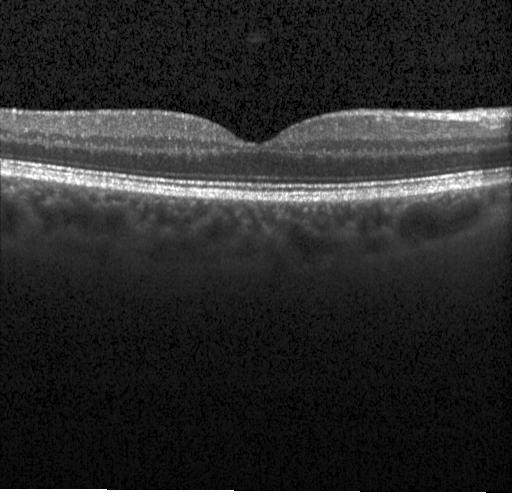
Optical coherence tomography scan. Heidelberg Spectralis OCT system. SD-OCT. Assessment: neither choroidal neovascularization, diabetic macular edema, nor drusen.